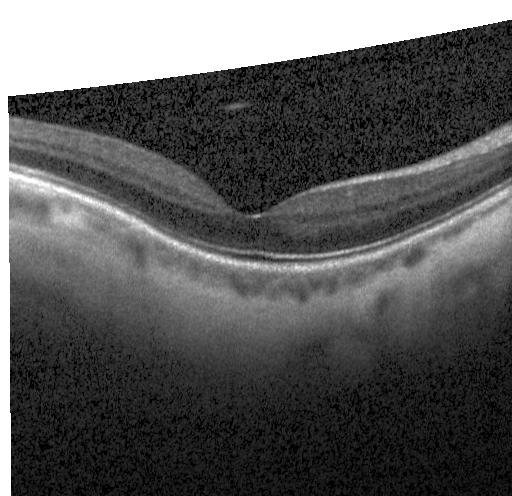 Retinal OCT B-scan — The scan shows no choroidal neovascularization, diabetic macular edema, or drusen.